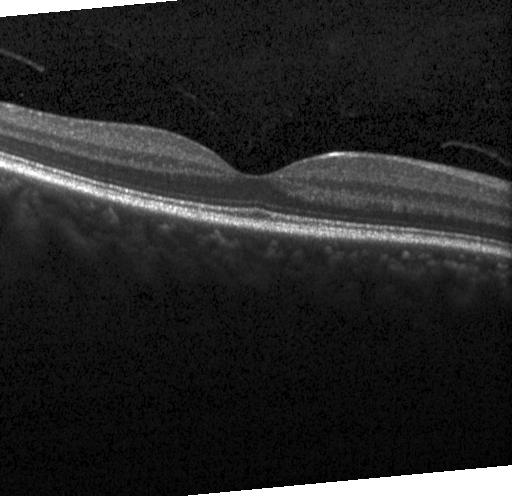
Horizontal scan through the fovea · optical coherence tomography scan. Assessment: no CNV, no DME, and no drusen.